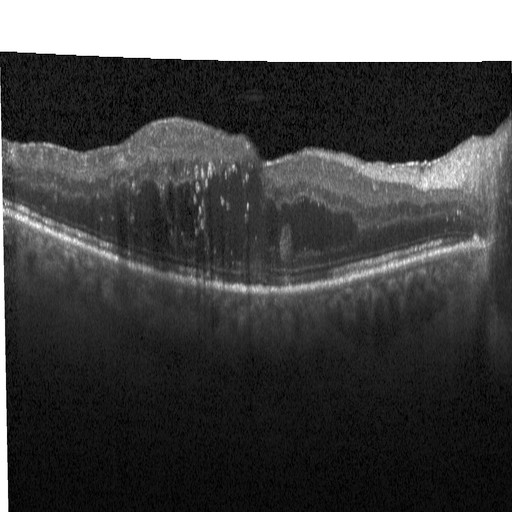
Heidelberg Spectralis. Retinal OCT cross-section. Macular OCT: diabetic macular edema (DME).